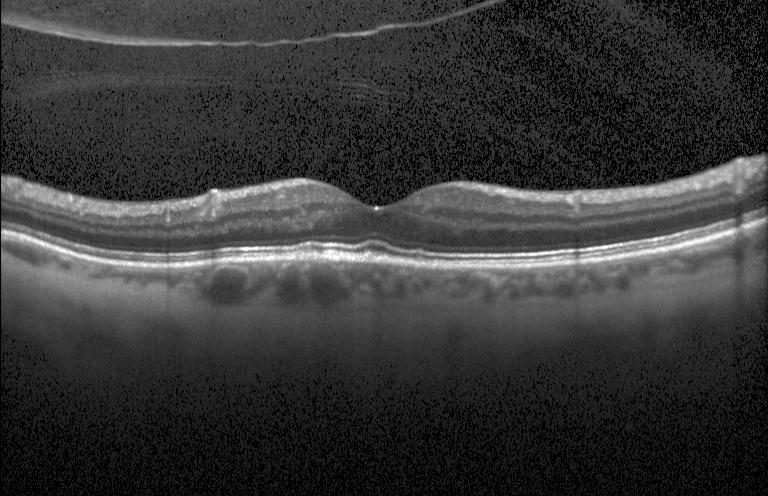

Retinal OCT cross-section showing sub-RPE drusenoid deposits.